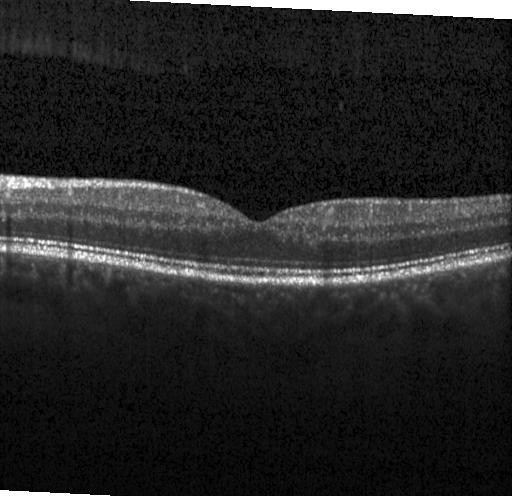

Retinal OCT cross-section showing neither choroidal neovascularization, diabetic macular edema, nor drusen.